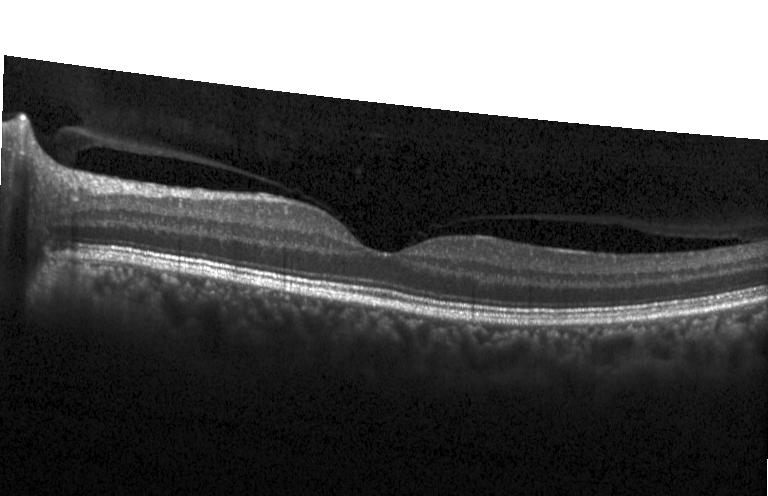 Macular OCT: no choroidal neovascularization, diabetic macular edema, or drusen.